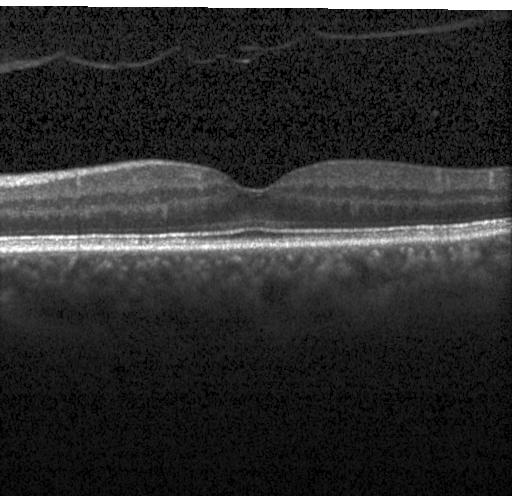 Optical coherence tomography B-scan
Diagnosis: no choroidal neovascularization, no diabetic macular edema, and no drusen.